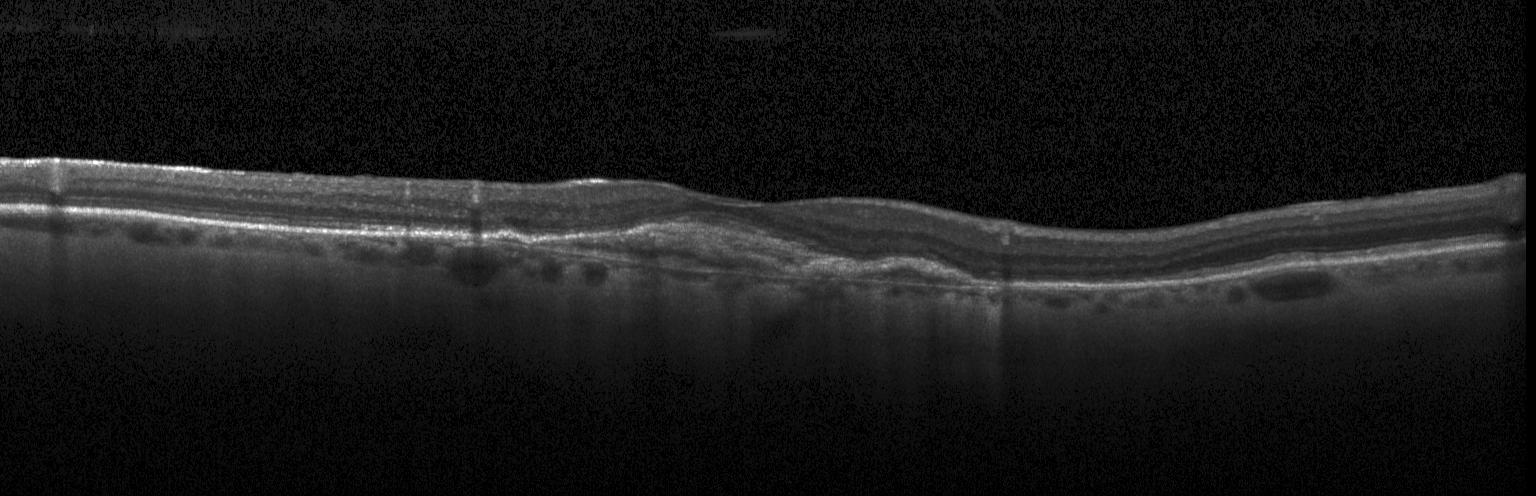
OCT line scan.
Macular OCT: CNV.